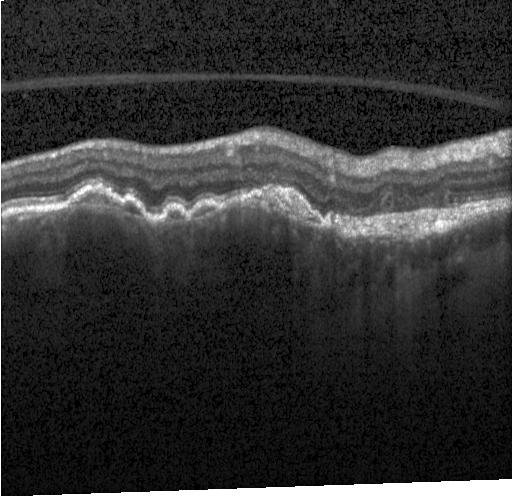 Fovea-centered. Spectral-domain OCT. Optical coherence tomography scan — Diagnosis: CNV.